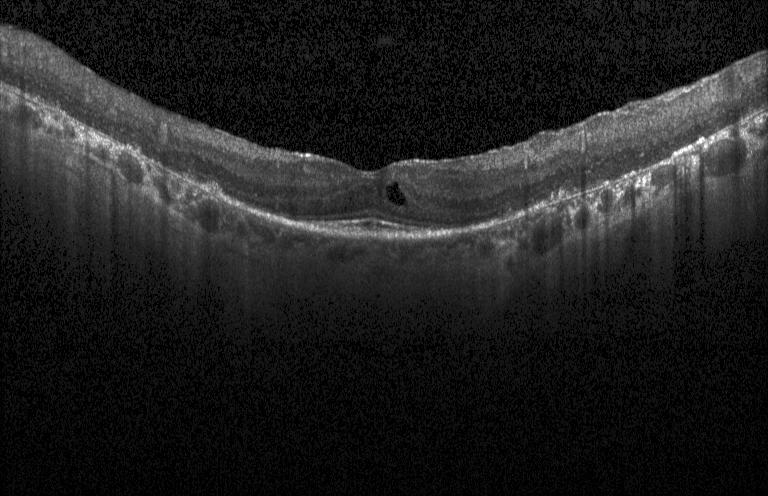 OCT B-scan; acquired on a Heidelberg Spectralis; fovea-centered. Diagnosis: DME.